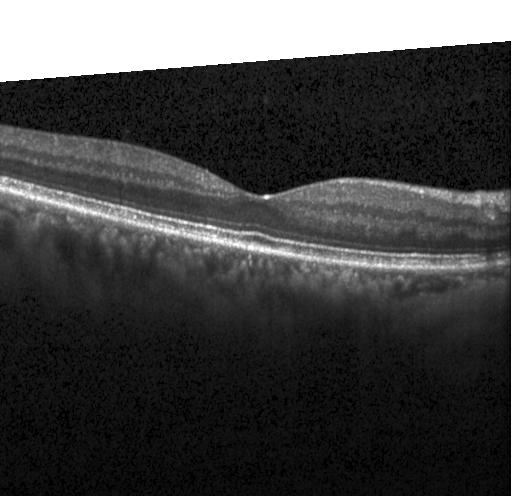

Acquired on a Heidelberg Spectralis · spectral-domain OCT · OCT B-scan. Finding: no choroidal neovascularization, diabetic macular edema, or drusen.